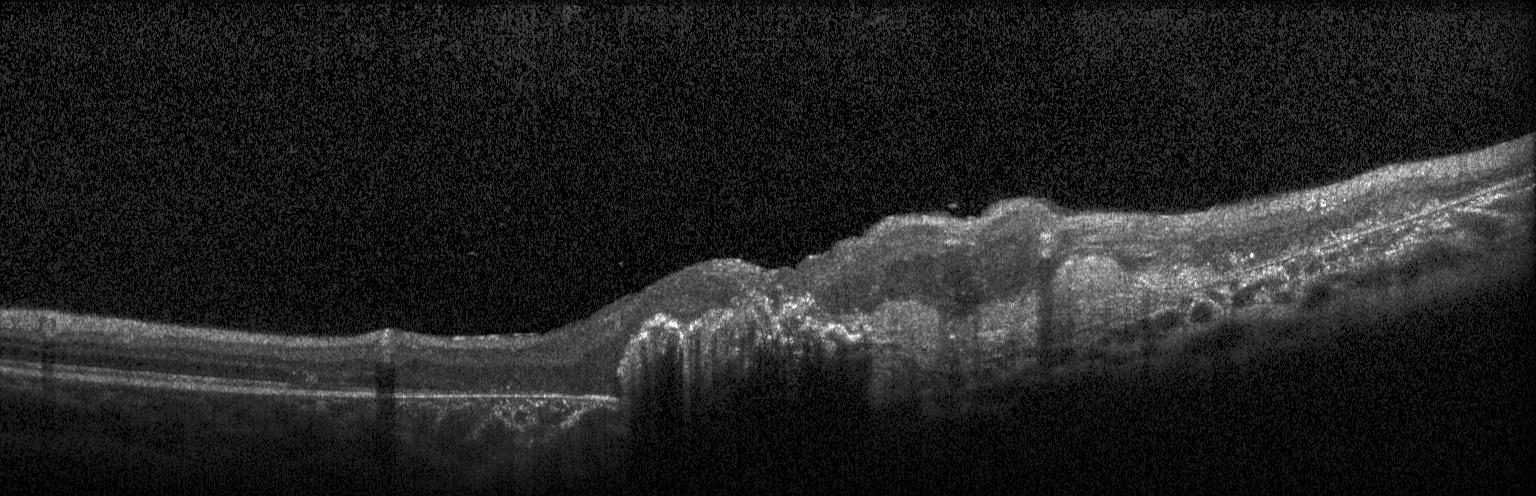 Spectral-domain optical coherence tomography; OCT B-scan; through the macula. CNV.